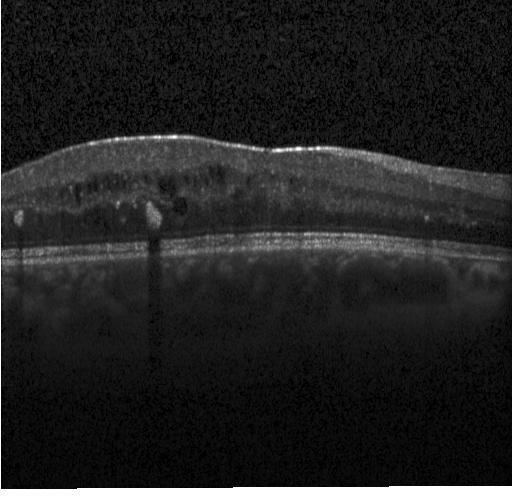

Acquired on a Heidelberg Spectralis, spectral-domain optical coherence tomography, OCT line scan, centered on the fovea. Impression: diabetic macular edema.